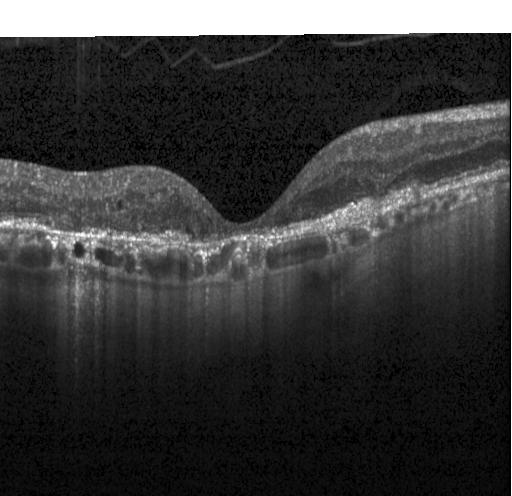

OCT line scan · SD-OCT · macular scan.
Assessment: choroidal neovascularization.